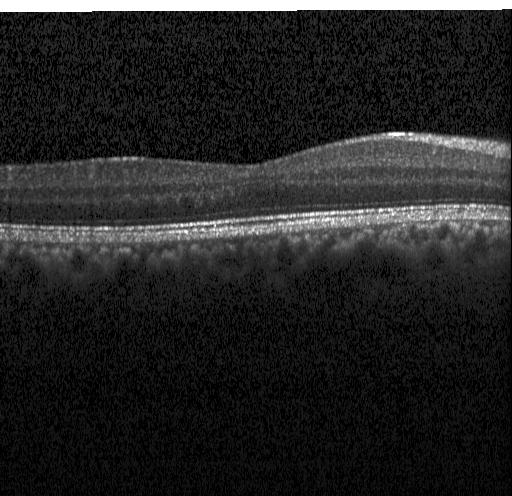
Assessment: no choroidal neovascularization, diabetic macular edema, or drusen.